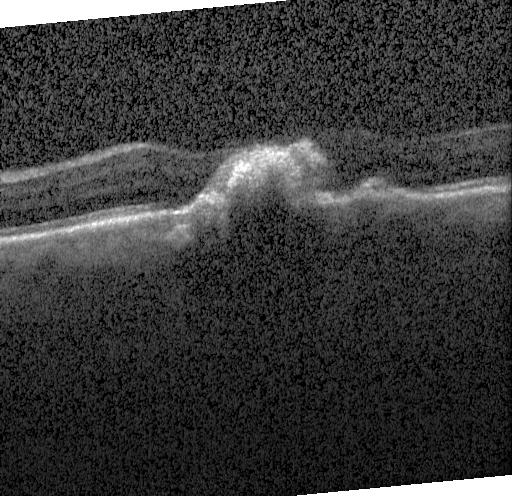

Heidelberg Spectralis; OCT line scan
Diagnosis: a choroidal neovascular membrane.